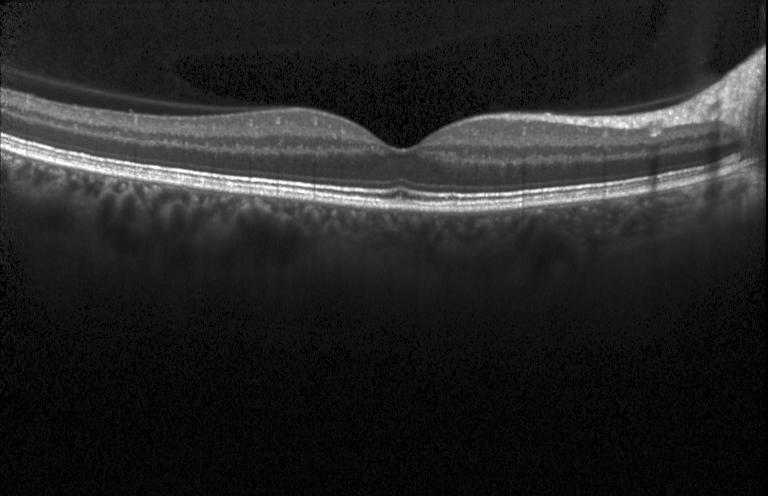 Acquired on a Heidelberg Spectralis. Retinal OCT cross-section
Impression: no CNV, no DME, and no drusen.